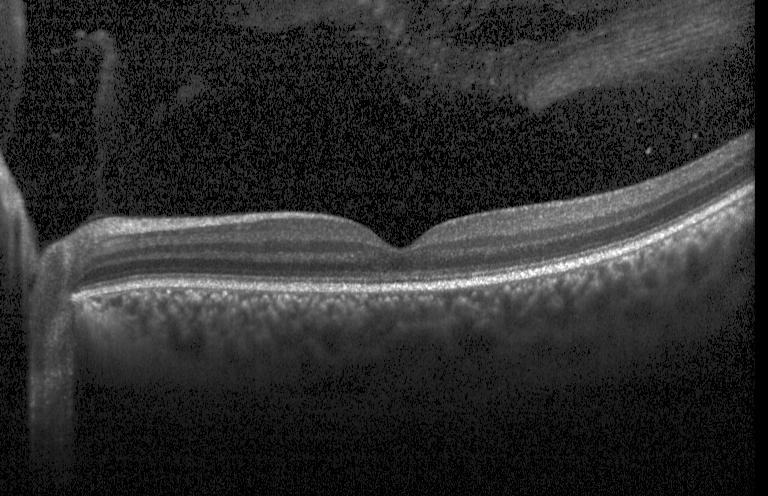
Dx: no choroidal neovascularization, no diabetic macular edema, and no drusen.